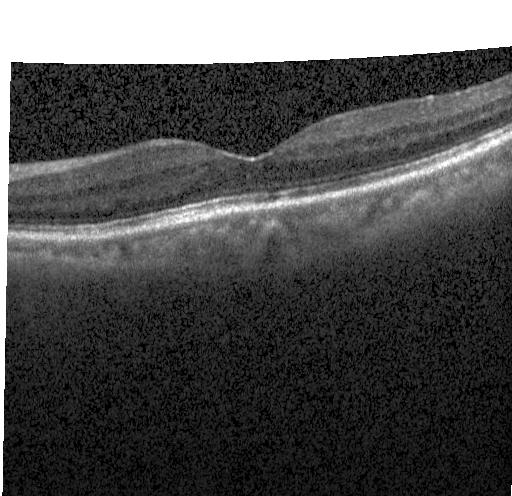

OCT line scan; horizontal scan through the fovea; SD-OCT. Assessment: no evidence of choroidal neovascularization, diabetic macular edema, or drusen.